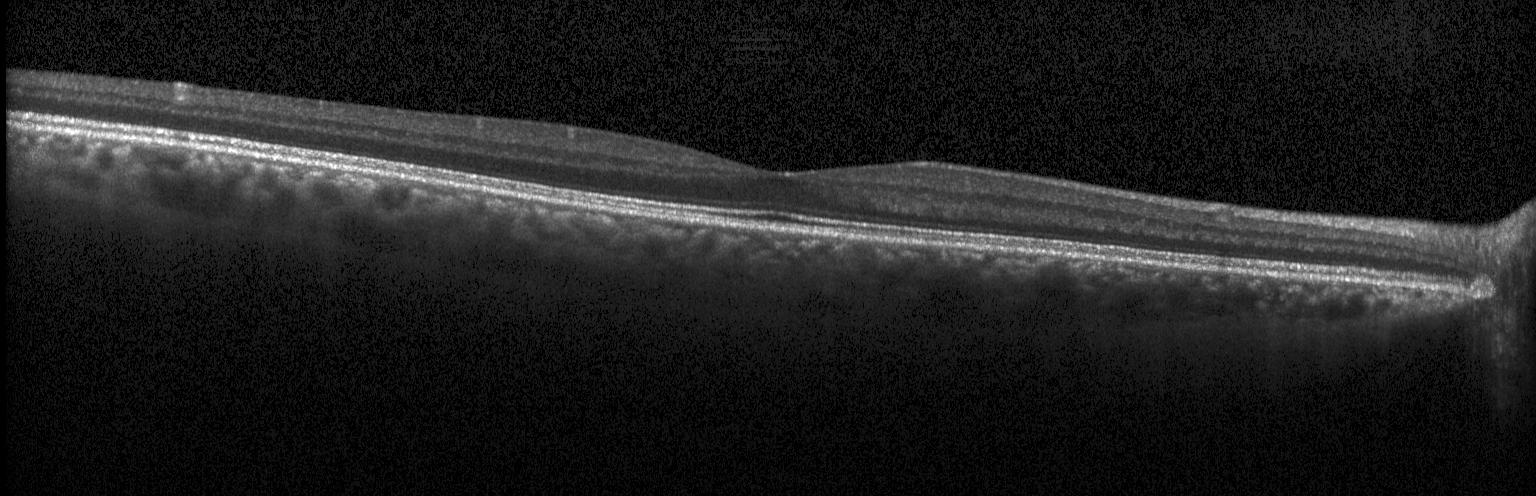 Heidelberg Spectralis, horizontal scan through the fovea, optical coherence tomography scan, SD-OCT
Diagnosis: no CNV, DME, or drusen.